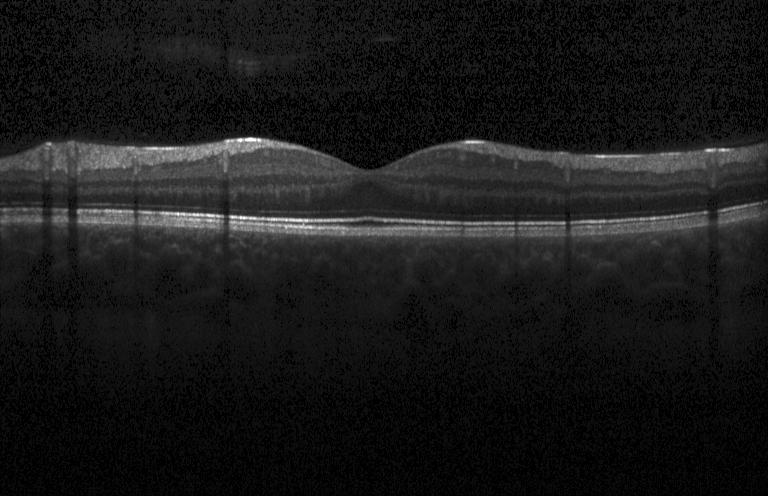 Spectral-domain OCT B-scan: neither choroidal neovascularization, diabetic macular edema, nor drusen.